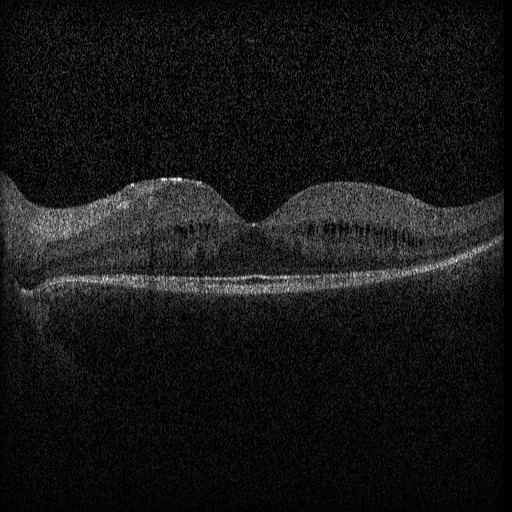
Heidelberg Spectralis OCT system · through the macula · optical coherence tomography B-scan. Finding: diabetic macular edema (DME).